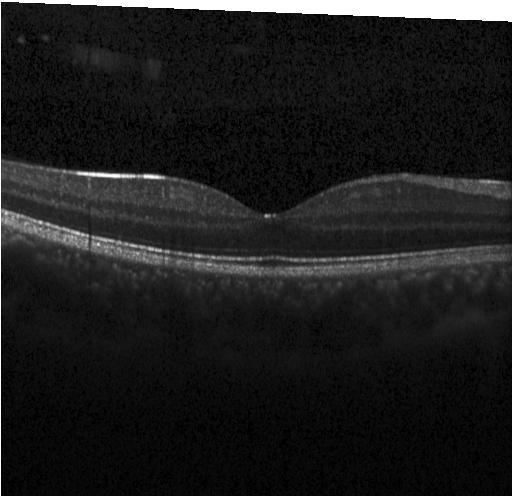 OCT finding: neither CNV, DME, nor drusen.